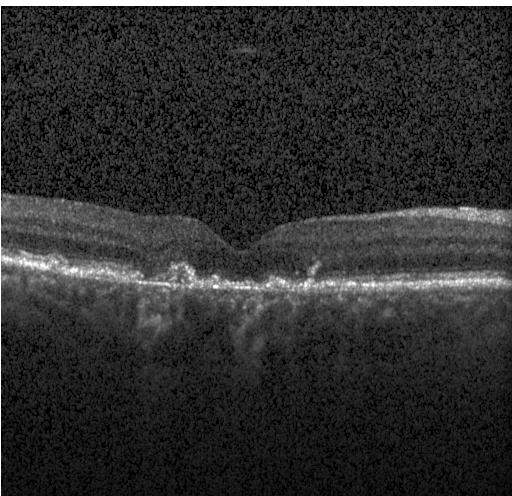

This B-scan demonstrates choroidal neovascularization.